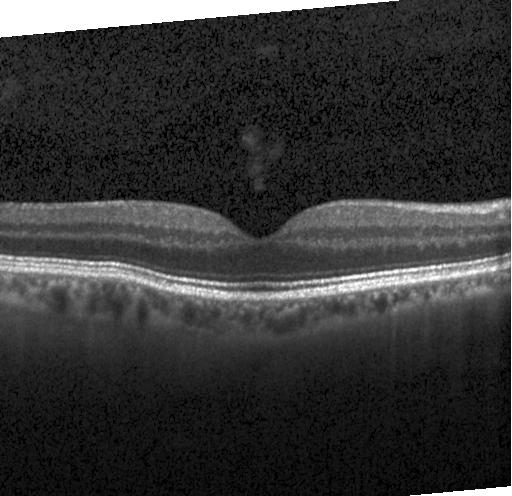

Spectral-domain OCT; retinal OCT B-scan
Diagnosis: no evidence of choroidal neovascularization, diabetic macular edema, or drusen.